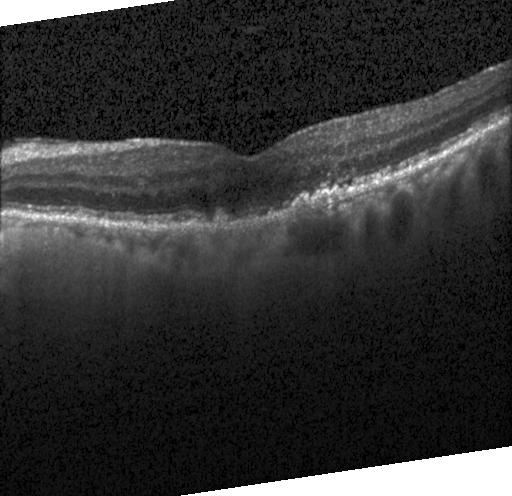

Dx: CNV.